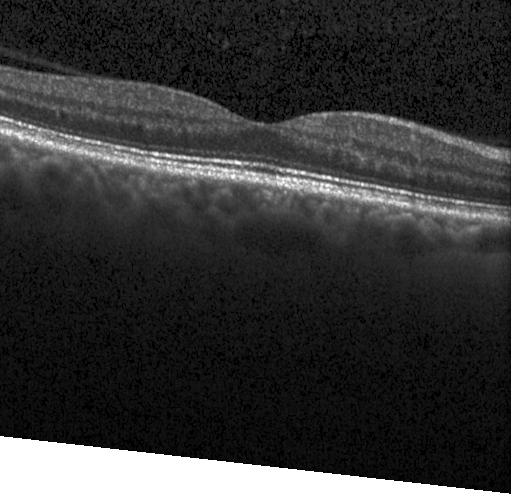

Heidelberg Spectralis OCT system, OCT B-scan, through the macula — Finding: neither choroidal neovascularization, diabetic macular edema, nor drusen.